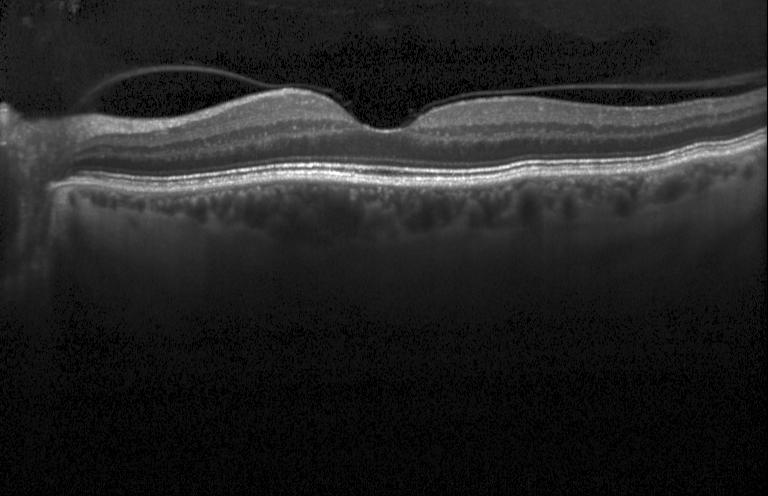

Spectral-domain OCT. Heidelberg Spectralis OCT system. Retinal OCT cross-section
Diagnosis: neither CNV, DME, nor drusen.